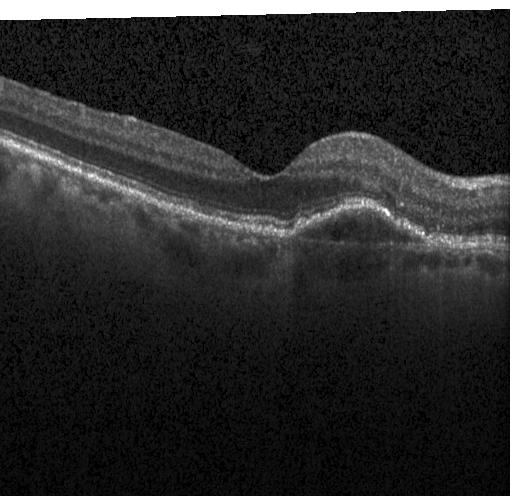

Macular OCT demonstrating CNV.